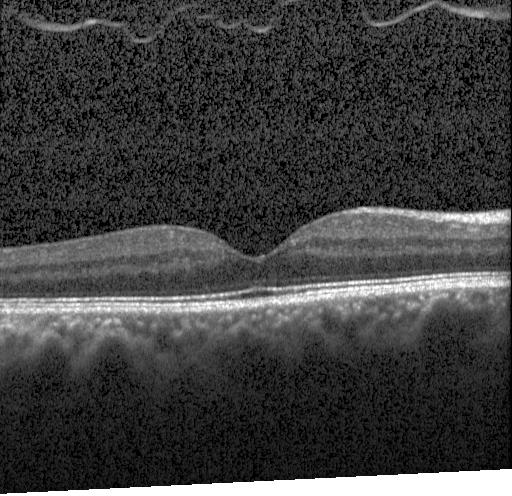

OCT finding: no choroidal neovascularization, no diabetic macular edema, and no drusen.